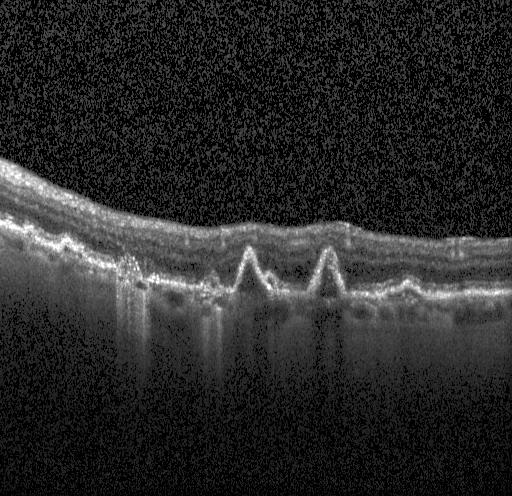

Optical coherence tomography B-scan · spectral-domain optical coherence tomography · horizontal scan through the fovea · instrument: Heidelberg Spectralis.
This B-scan demonstrates choroidal neovascularization.